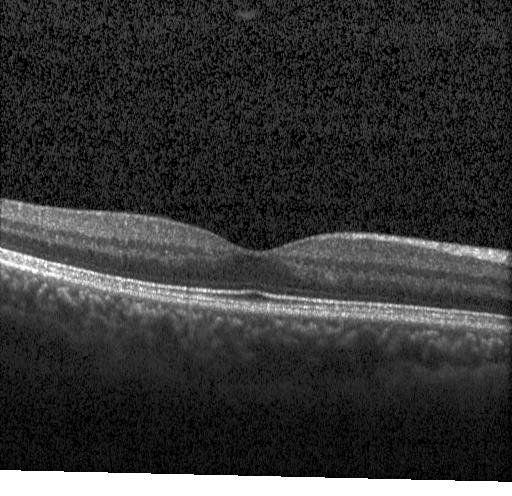

Macular OCT demonstrating no choroidal neovascularization, diabetic macular edema, or drusen.